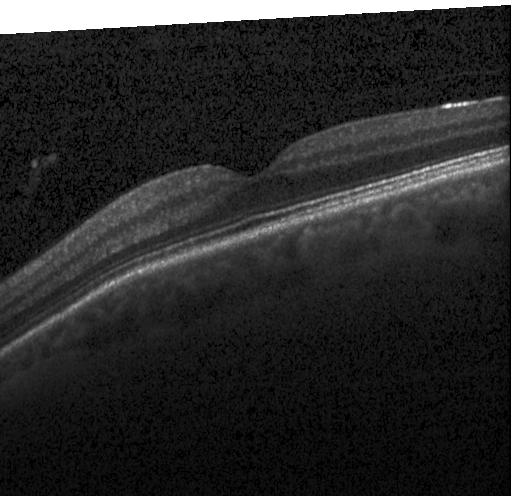 Optical coherence tomography scan. Spectral-domain OCT. OCT finding: neither CNV, DME, nor drusen.